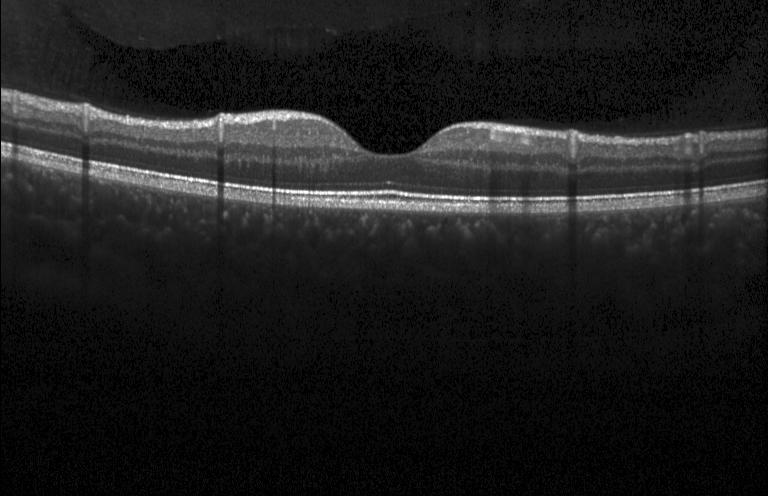

Finding: no choroidal neovascularization, no diabetic macular edema, and no drusen.